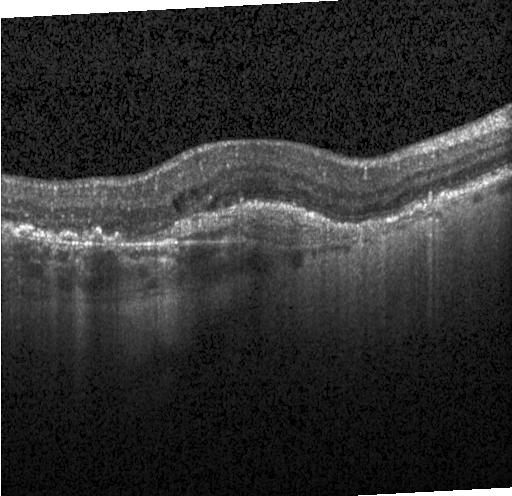 OCT scan showing choroidal neovascularization (CNV).